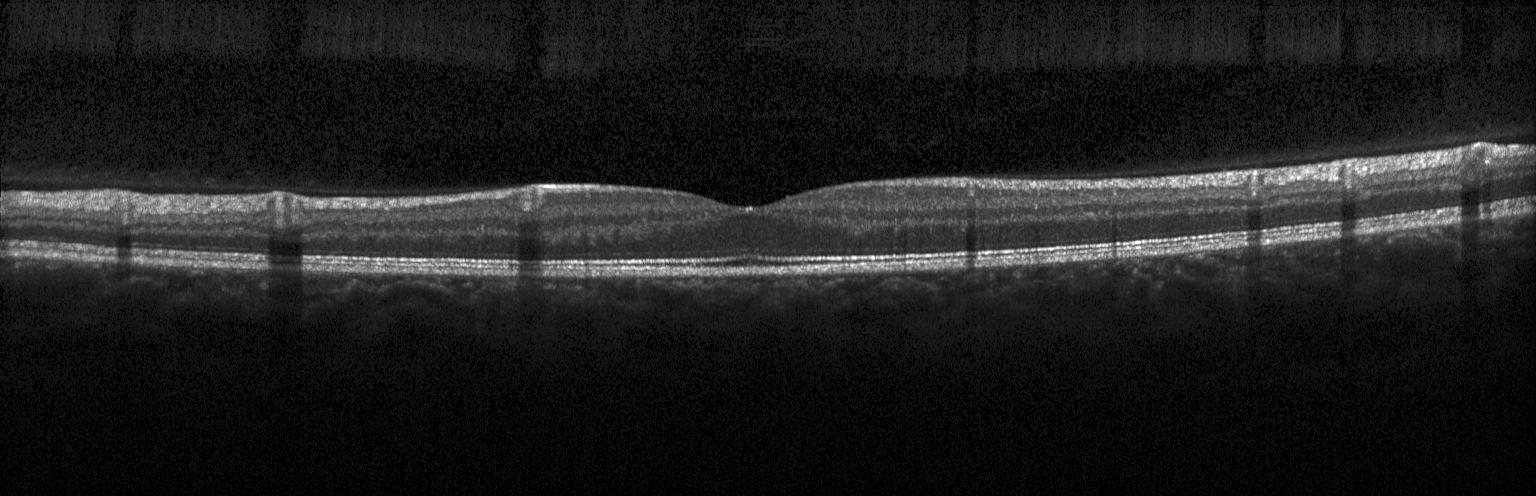

Macular scan, spectral-domain OCT, retinal OCT B-scan — Impression: no choroidal neovascularization, no diabetic macular edema, and no drusen.